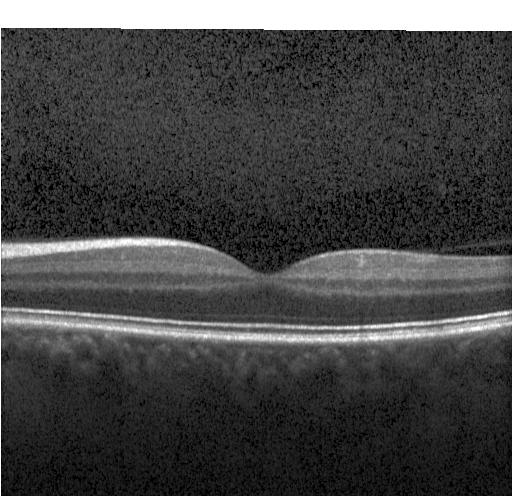 Macular scan. OCT B-scan. Instrument: Heidelberg Spectralis. Spectral-domain OCT. This B-scan demonstrates no choroidal neovascularization, no diabetic macular edema, and no drusen.